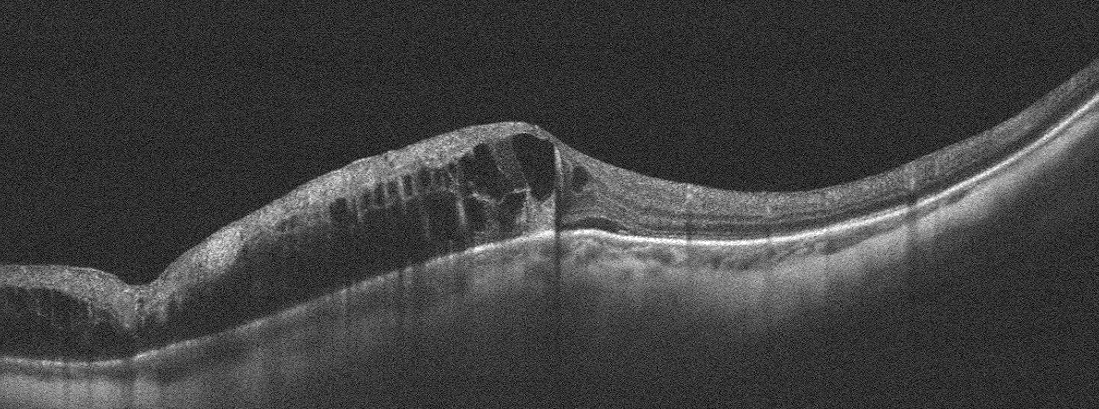 OCT B-scan — Diagnosis: RVO.